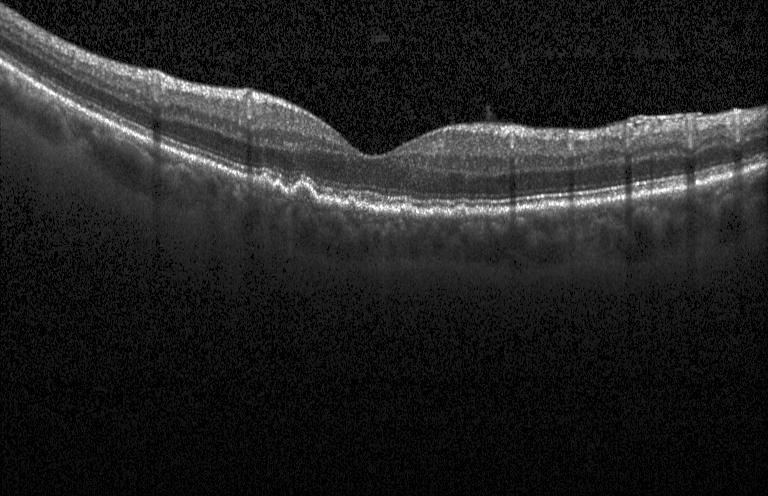 Dx: multiple drusen.